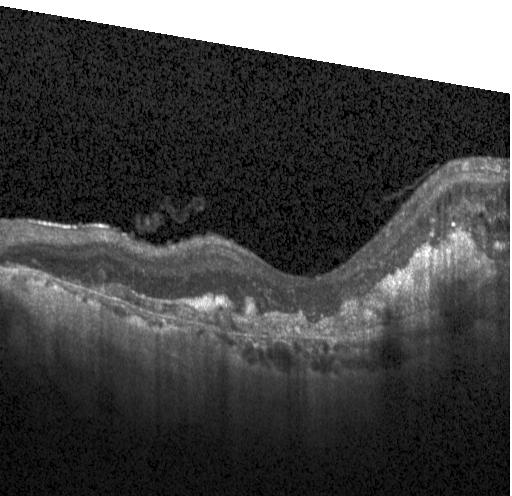

OCT line scan. Assessment: choroidal neovascularization (CNV).